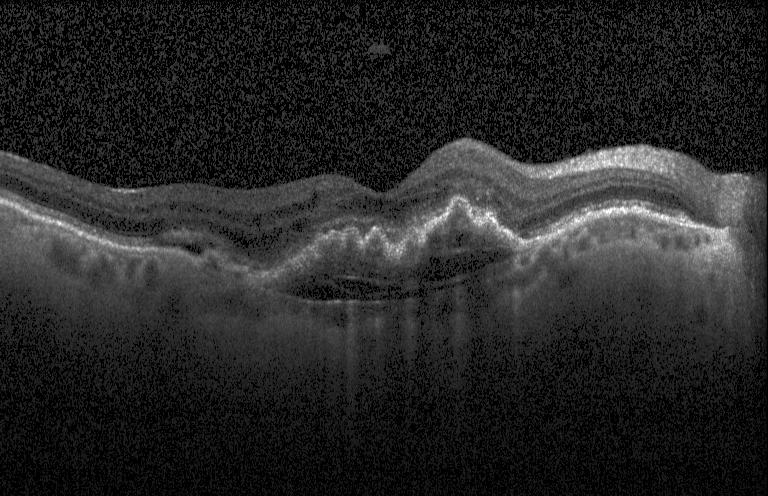
Through the macula; spectral-domain OCT; optical coherence tomography B-scan
Impression: a choroidal neovascular membrane.